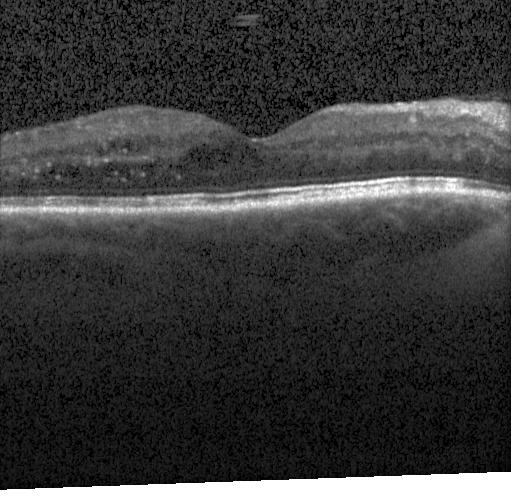 Diagnosis: diabetic macular edema.